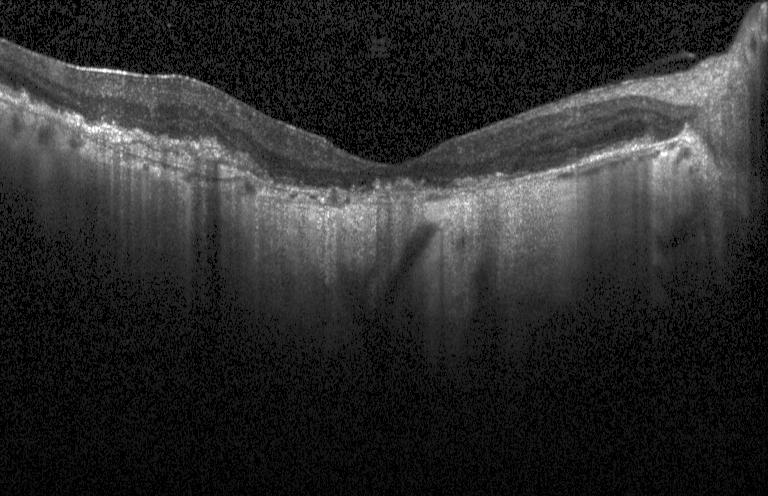
Macular scan · SD-OCT · instrument: Heidelberg Spectralis · OCT B-scan — Finding: choroidal neovascularization (CNV).